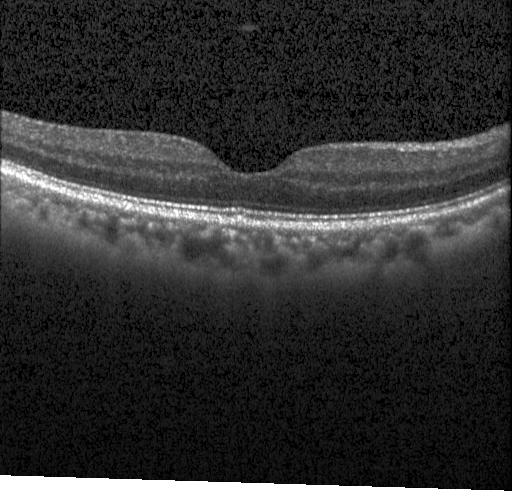
Centered on the fovea; spectral-domain OCT; OCT B-scan; Heidelberg Spectralis OCT system.
Macular OCT: no evidence of choroidal neovascularization, diabetic macular edema, or drusen.